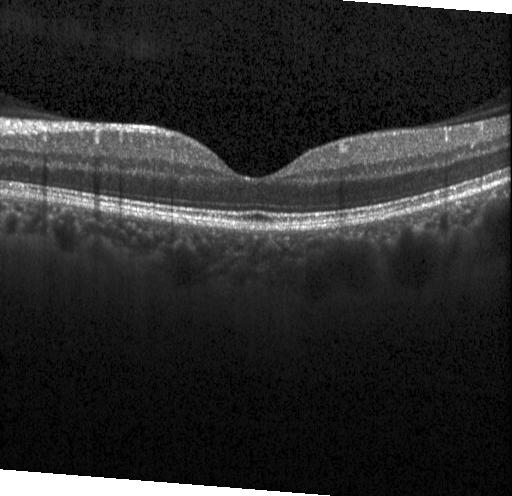
Diagnosis: no choroidal neovascularization, diabetic macular edema, or drusen.